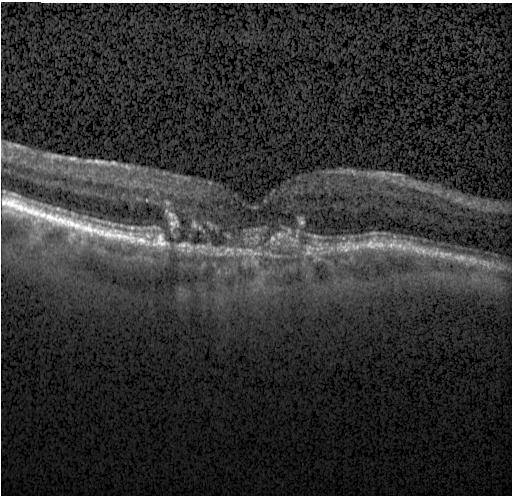
OCT scan showing choroidal neovascularization (CNV).